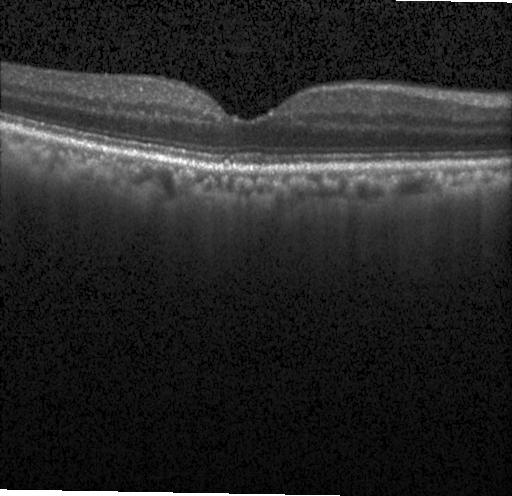 Optical coherence tomography B-scan.
Finding: no choroidal neovascularization, diabetic macular edema, or drusen.